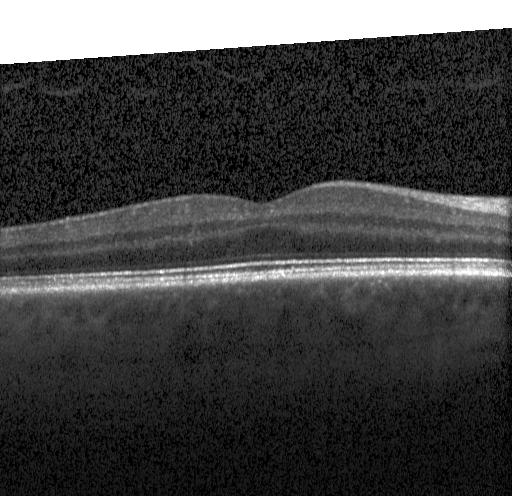 Retinal OCT cross-section · SD-OCT.
The scan shows no evidence of choroidal neovascularization, diabetic macular edema, or drusen.